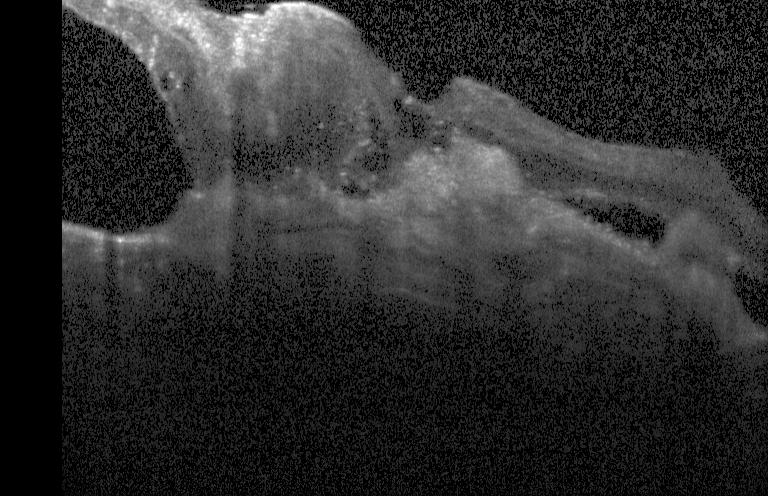
OCT B-scan · spectral-domain optical coherence tomography · acquired on a Heidelberg Spectralis · through the macula — Assessment: choroidal neovascularization.